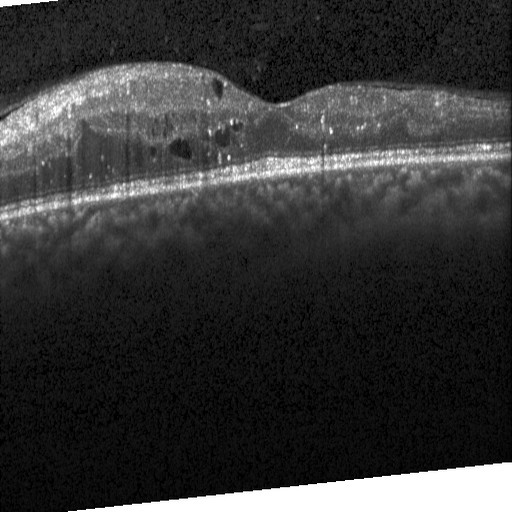 OCT B-scan
The scan shows diabetic macular edema (DME).